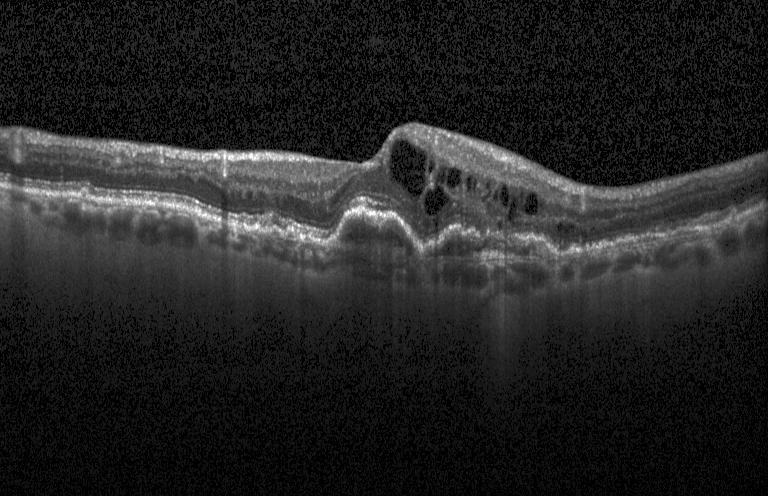
Diagnosis: a choroidal neovascular membrane.